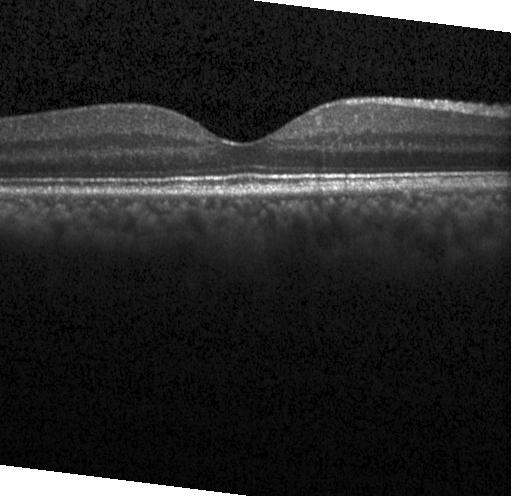

Optical coherence tomography scan.
Assessment: no CNV, DME, or drusen.